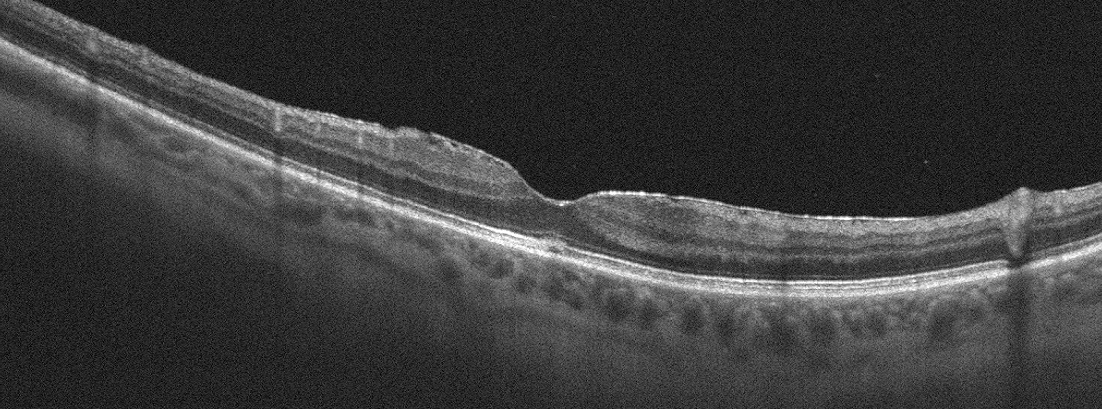 Retinal OCT cross-section. Macular OCT: epiretinal membrane (ERM).